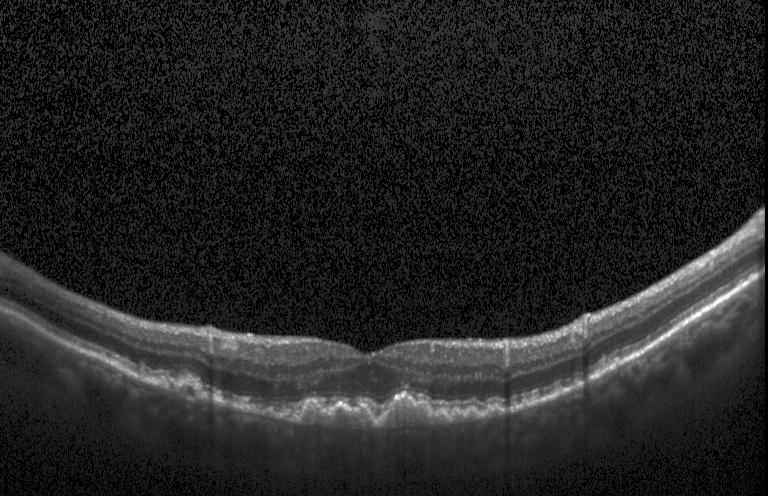 Macular OCT demonstrating drusen.